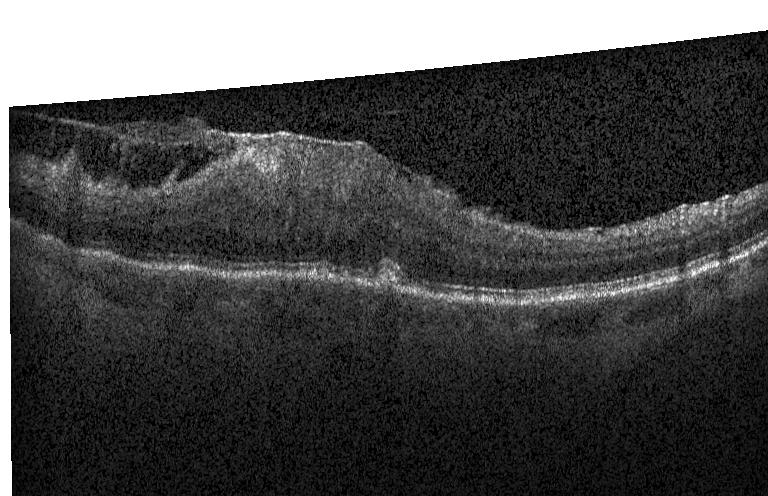

Dx: drusen.